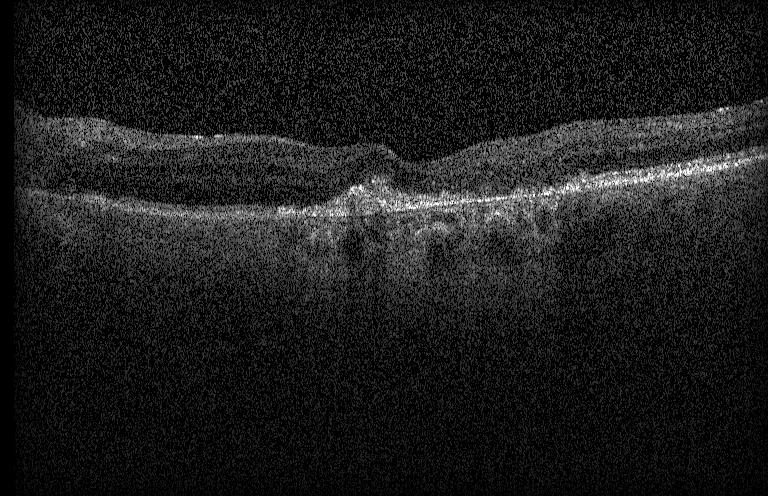
Optical coherence tomography scan.
Impression: choroidal neovascularization (CNV).